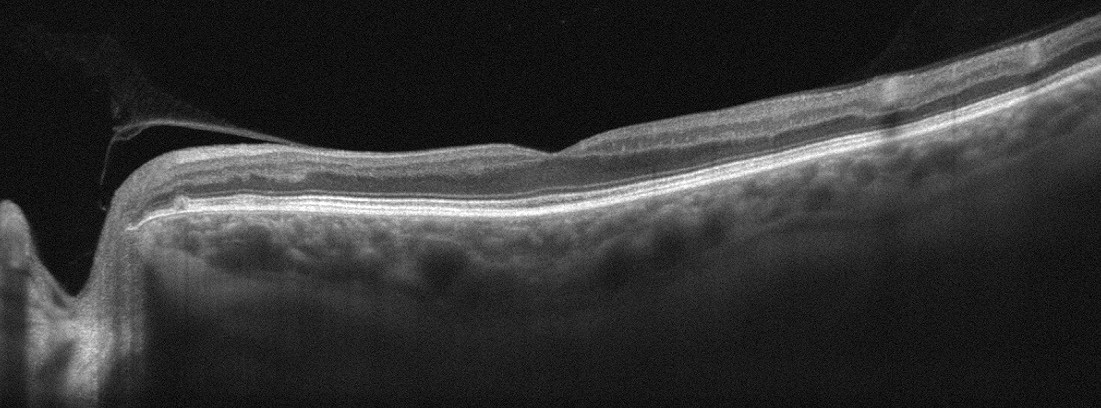

Retinal OCT cross-section
Impression: RVO.